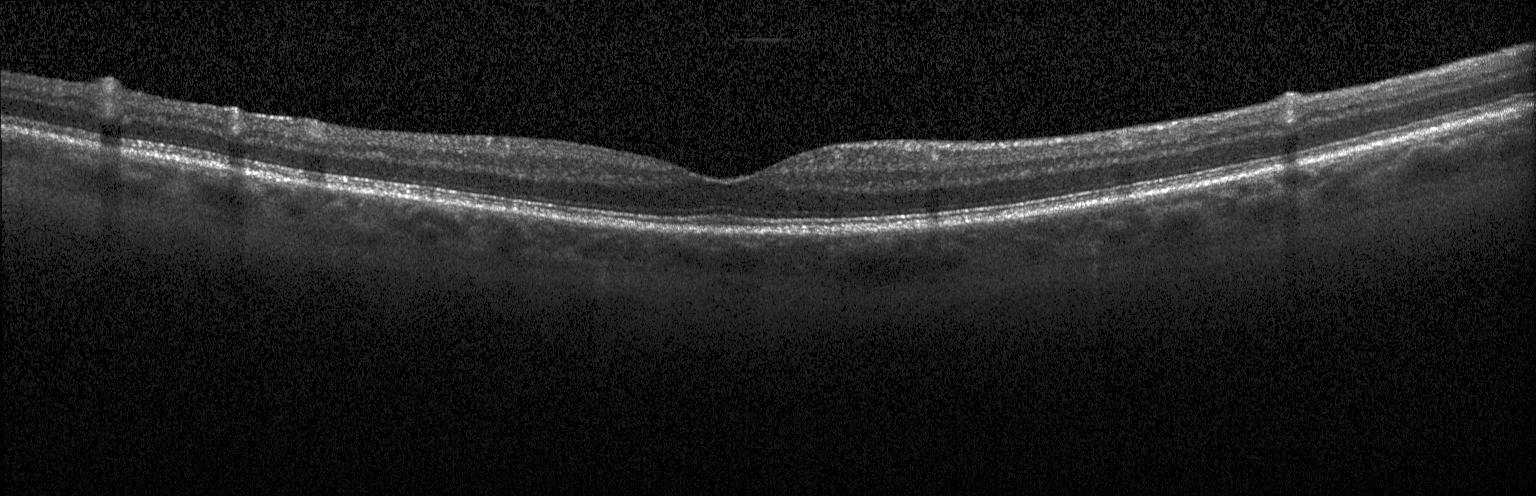
Diagnosis: neither CNV, DME, nor drusen.